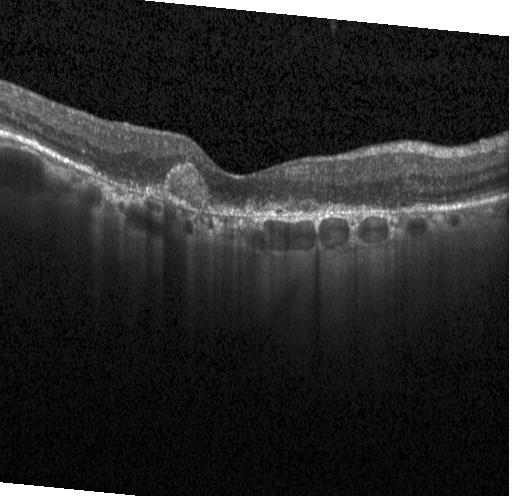 Optical coherence tomography B-scan · SD-OCT · Heidelberg Spectralis.
Finding: CNV.